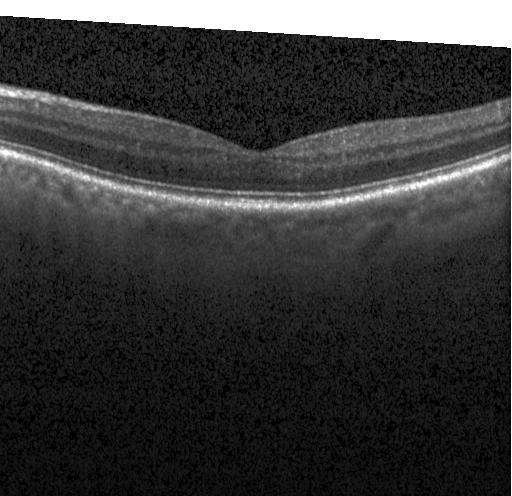 Heidelberg Spectralis, OCT B-scan, centered on the fovea, SD-OCT — Macular OCT: no CNV, DME, or drusen.